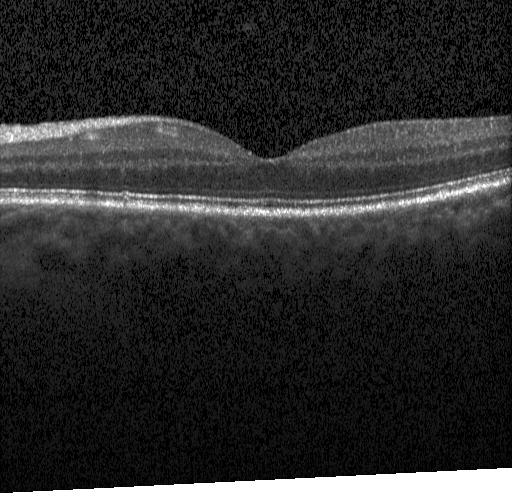 Instrument: Heidelberg Spectralis · spectral-domain OCT · optical coherence tomography scan — Diagnosis: neither choroidal neovascularization, diabetic macular edema, nor drusen.